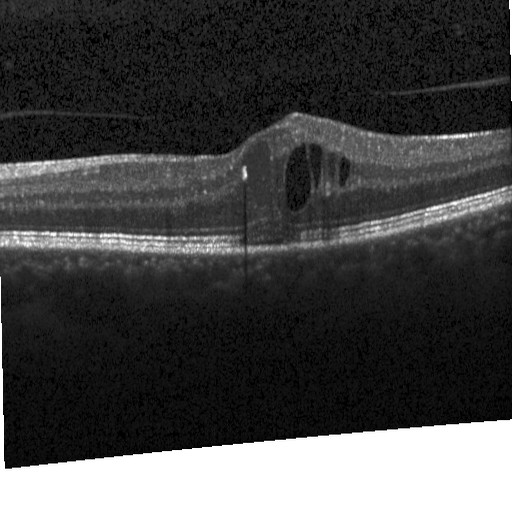

Impression: diabetic macular edema.